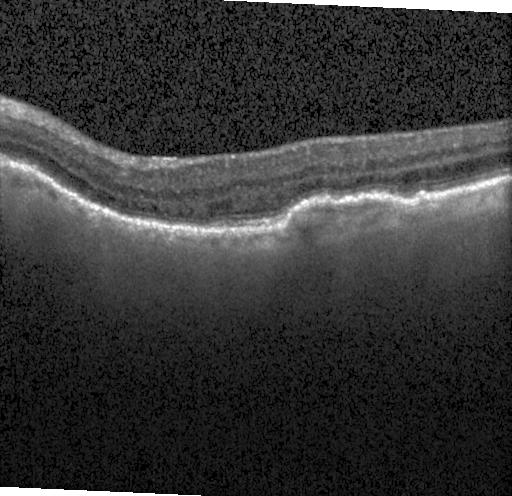

Optical coherence tomography scan
This B-scan demonstrates a choroidal neovascular membrane.